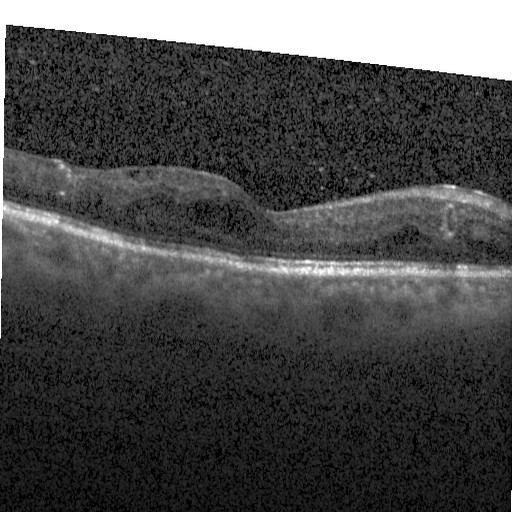 OCT B-scan showing diabetic macular edema (DME).